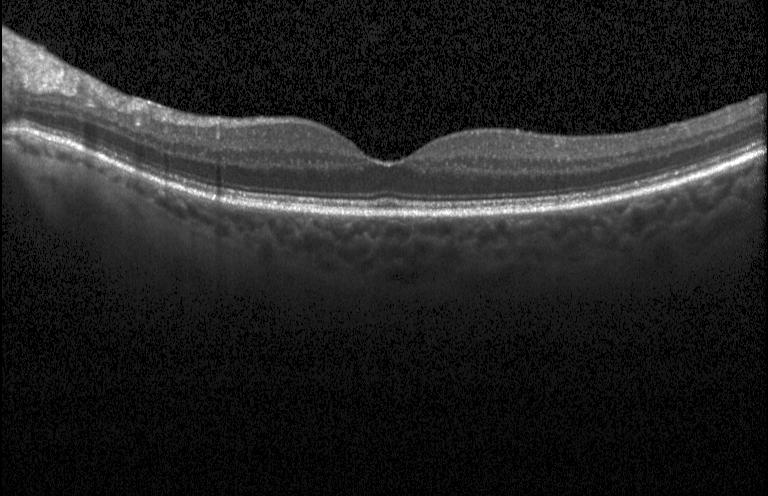 Spectral-domain optical coherence tomography, Heidelberg Spectralis, optical coherence tomography scan, through the macula.
OCT finding: no evidence of choroidal neovascularization, diabetic macular edema, or drusen.